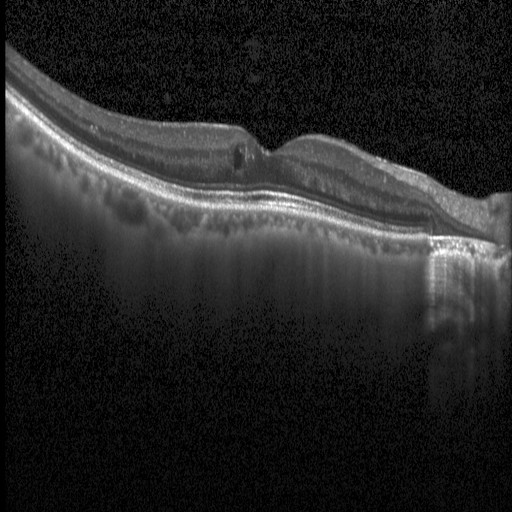 The scan shows DME.